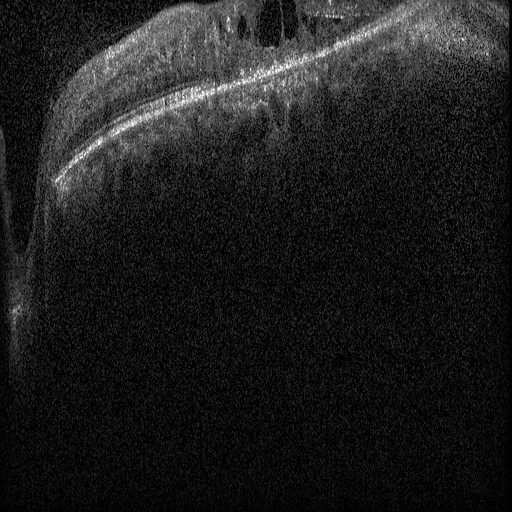 Finding: DME.